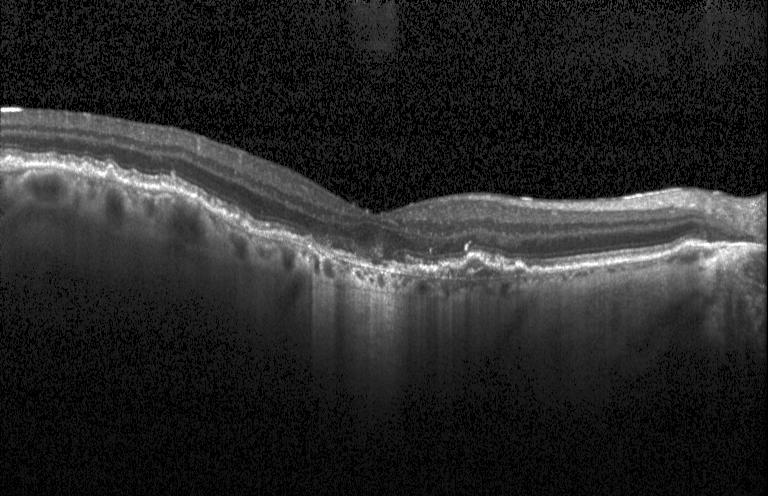 Centered on the fovea; retinal OCT B-scan. Finding: a choroidal neovascular membrane.